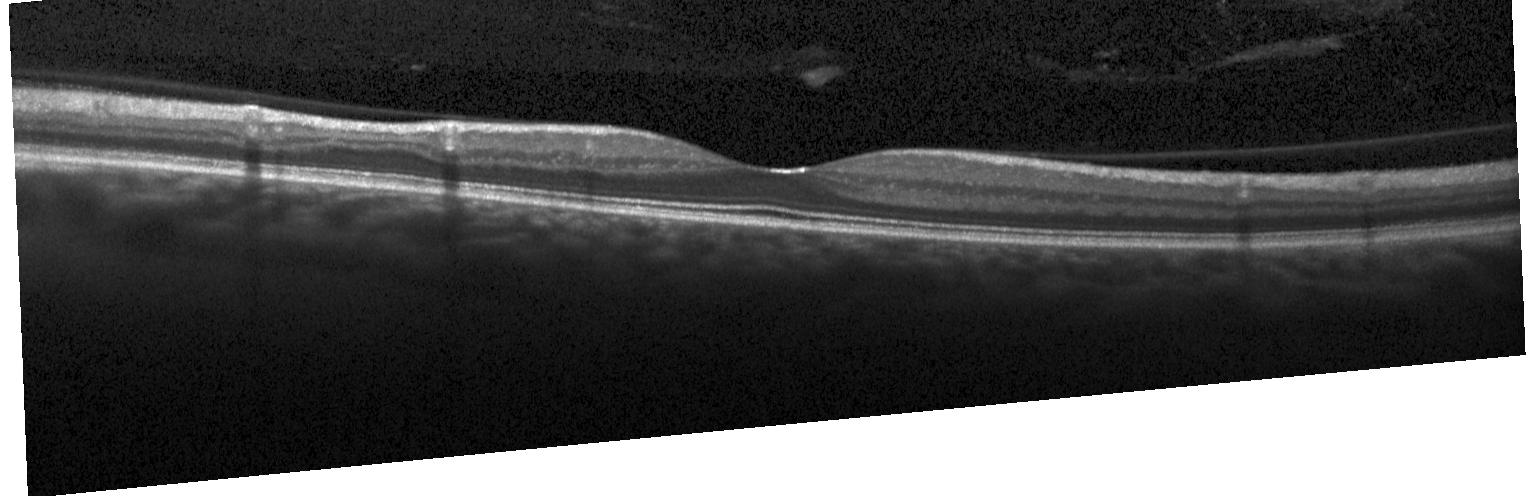
Spectral-domain OCT. Fovea-centered. Retinal OCT cross-section — Diagnosis: no choroidal neovascularization, diabetic macular edema, or drusen.